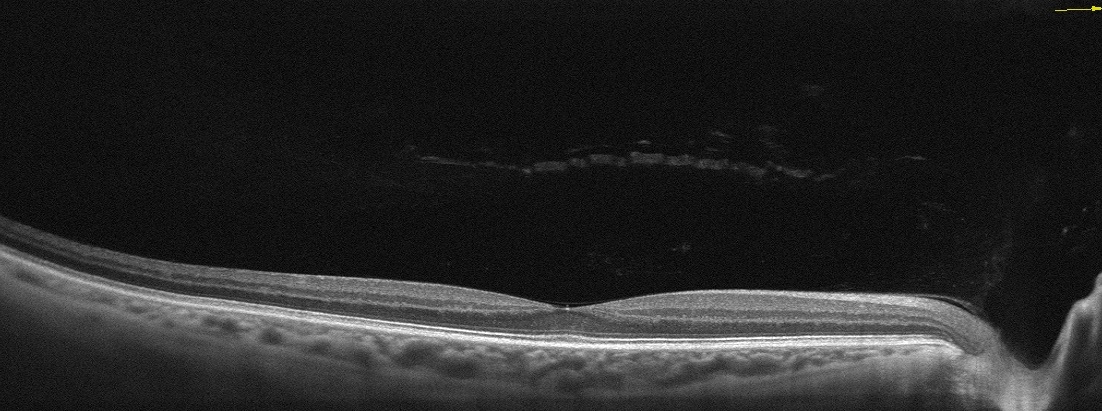
Optical coherence tomography scan, macular scan, Optovue Avanti RTVue XR. Impression: no AMD, DME, ERM, RAO, RVO, or VID.